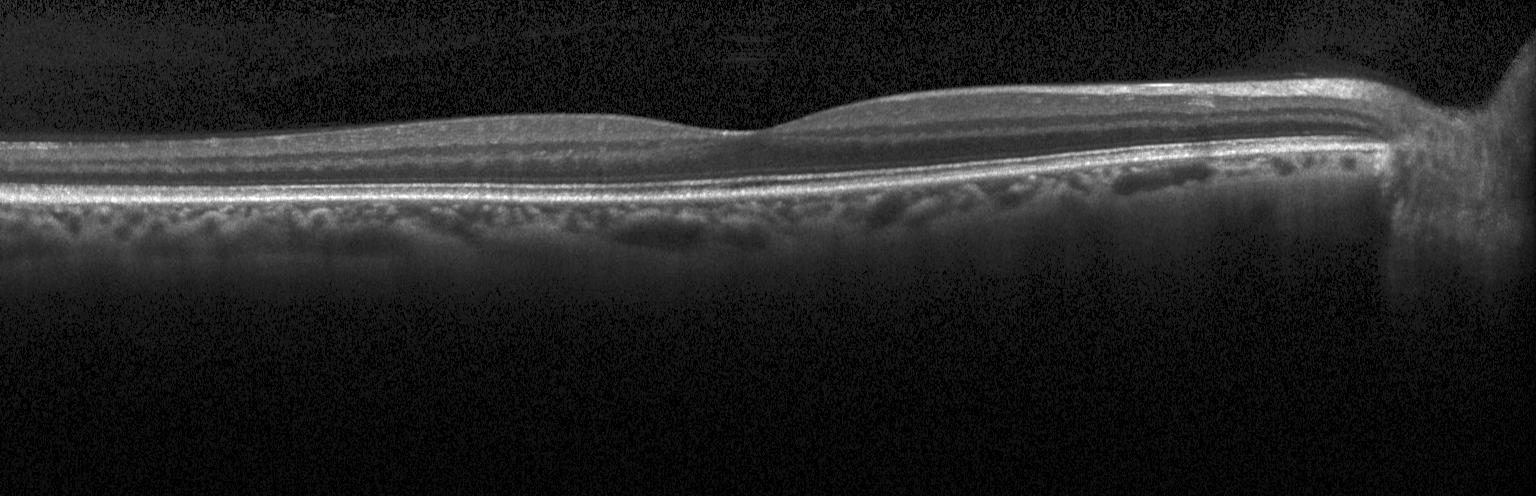

Spectral-domain OCT, OCT B-scan
Finding: no CNV, DME, or drusen.